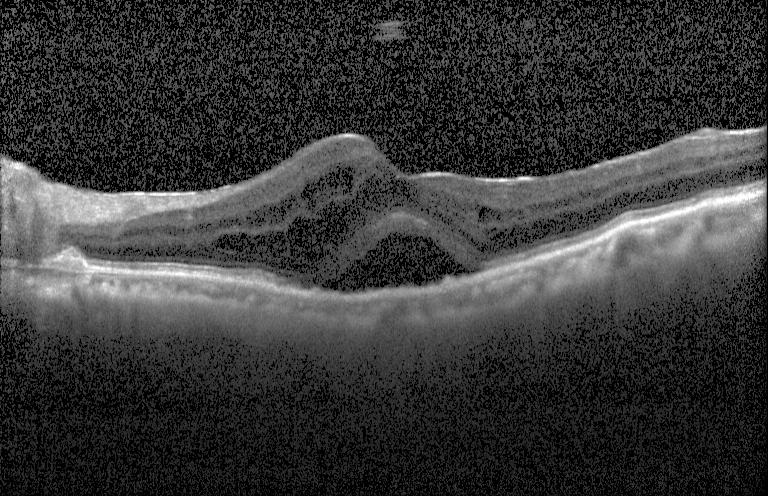

Assessment: diabetic macular edema (DME).